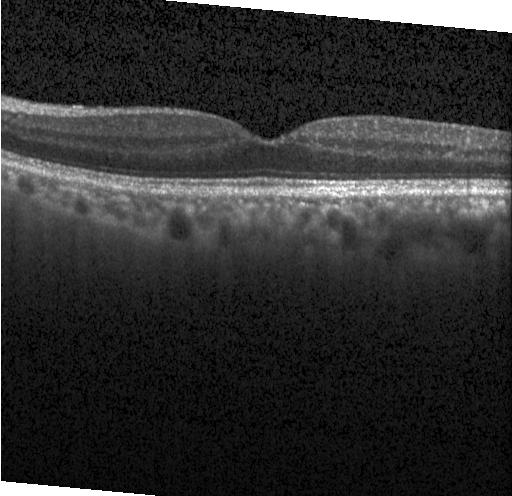 Diagnosis: no evidence of choroidal neovascularization, diabetic macular edema, or drusen.